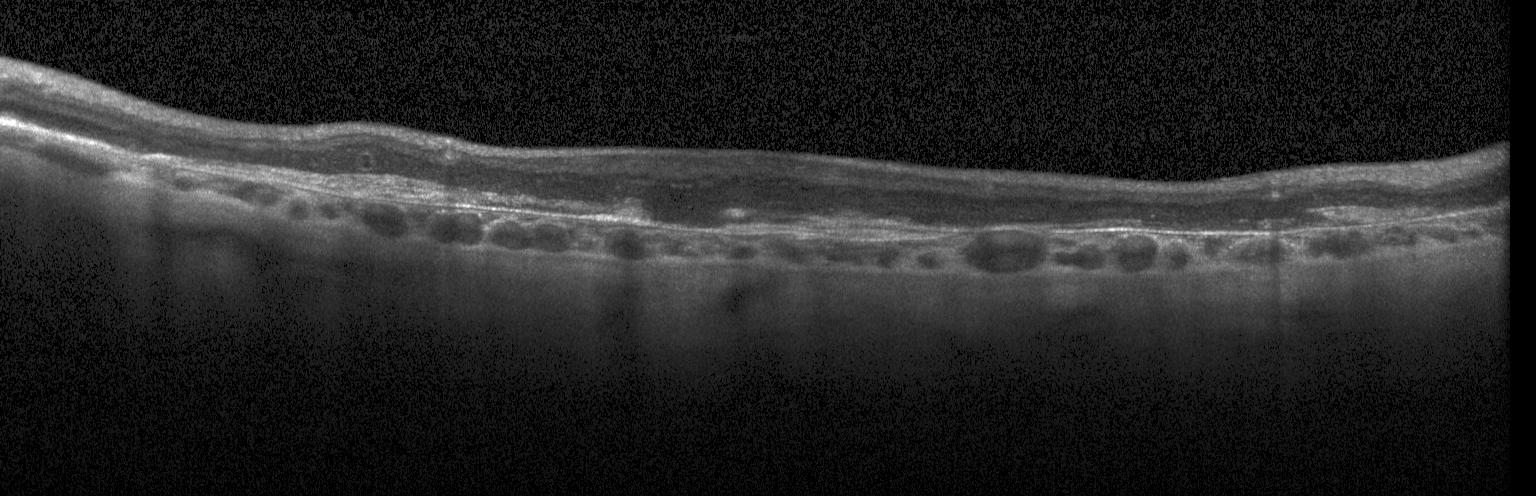

Horizontal scan through the fovea, instrument: Heidelberg Spectralis, spectral-domain OCT, retinal OCT cross-section — Impression: choroidal neovascularization.